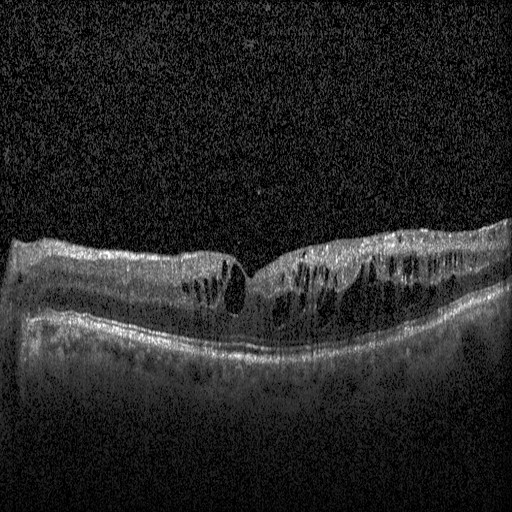

Retinal OCT cross-section; instrument: Heidelberg Spectralis; SD-OCT; macular scan — Diagnosis: diabetic macular edema.